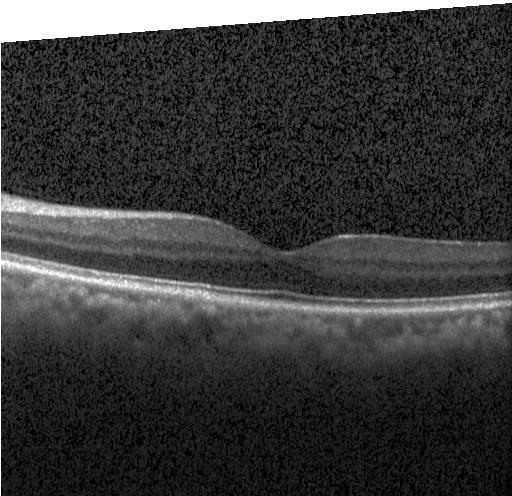
Optical coherence tomography B-scan.
Finding: neither choroidal neovascularization, diabetic macular edema, nor drusen.